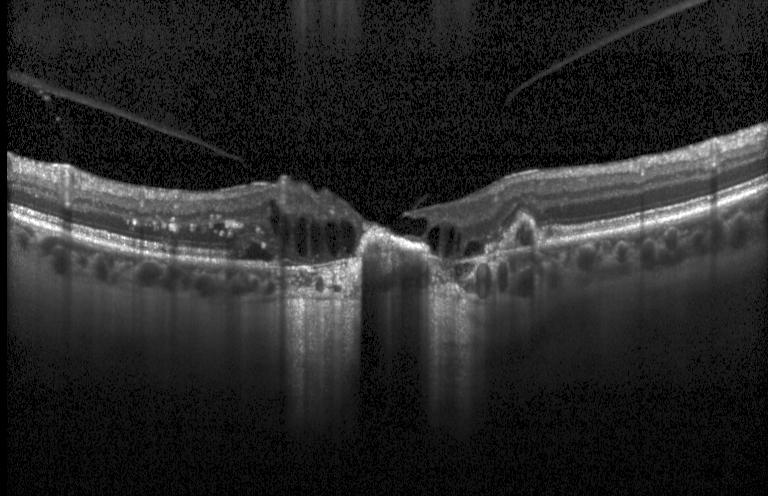

Retinal OCT cross-section; through the macula.
Finding: a choroidal neovascular membrane.